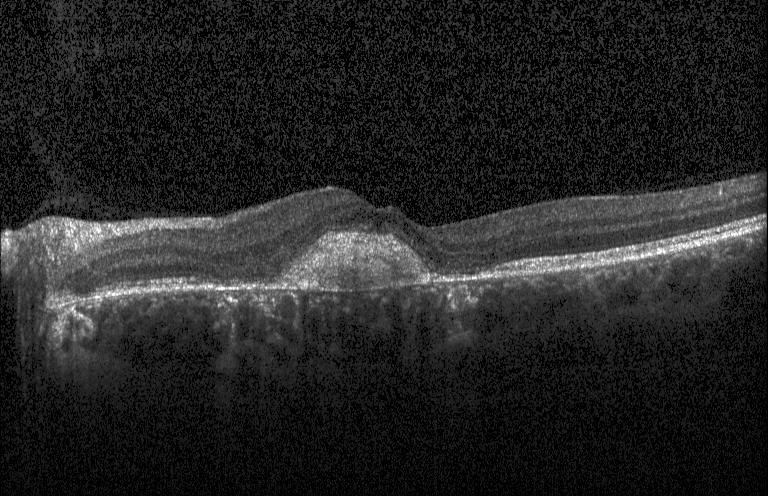

Acquired on a Heidelberg Spectralis. Centered on the fovea. Spectral-domain OCT. Retinal OCT cross-section.
Dx: choroidal neovascularization (CNV).